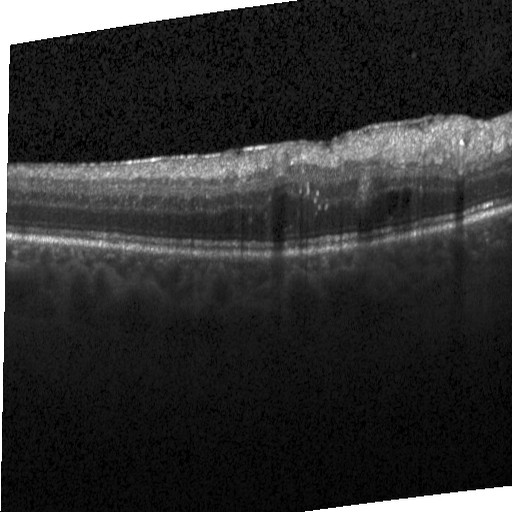

Optical coherence tomography scan. Horizontal scan through the fovea. Spectral-domain OCT. Heidelberg Spectralis.
Finding: diabetic macular edema.